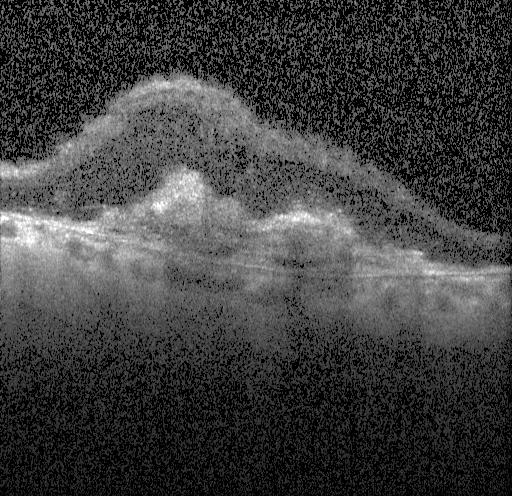

Spectral-domain OCT B-scan: a choroidal neovascular membrane.